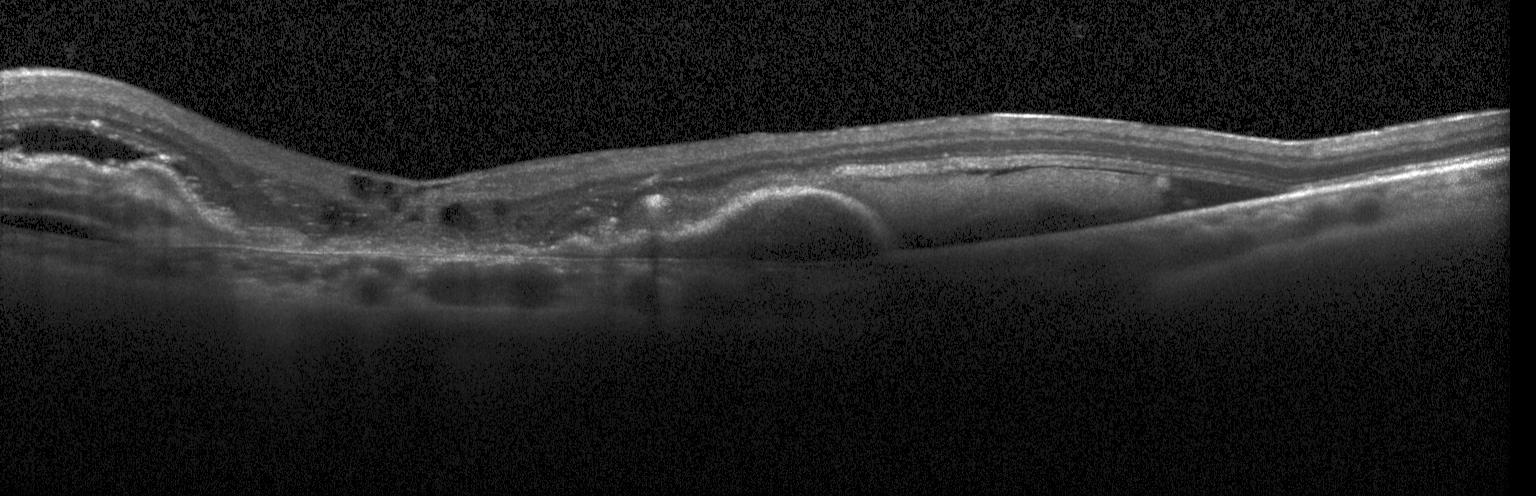
Macular scan; OCT B-scan.
Macular OCT: CNV.